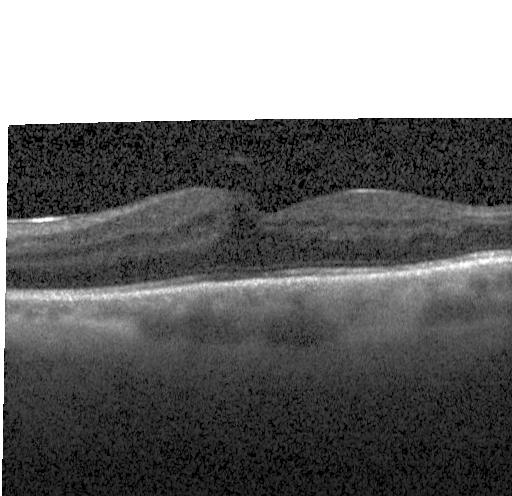

Spectral-domain optical coherence tomography; macular scan; OCT line scan; acquired on a Heidelberg Spectralis
Dx: DME.